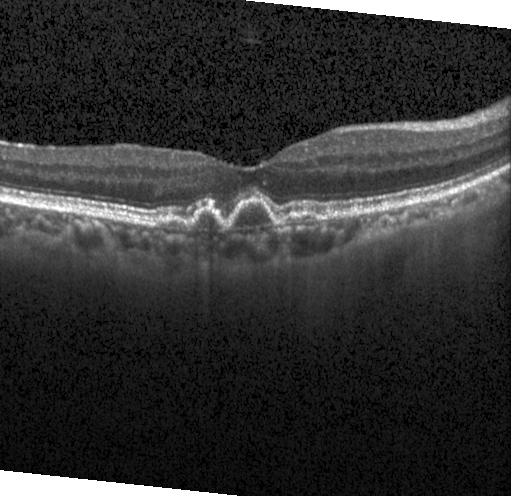
Spectral-domain OCT; Heidelberg Spectralis OCT system; optical coherence tomography B-scan — Diagnosis: a choroidal neovascular membrane.